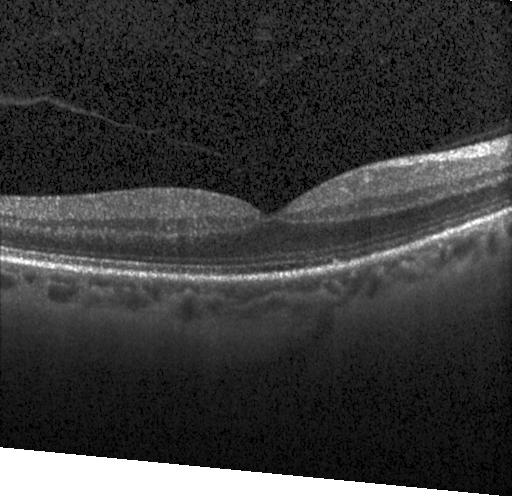

Spectral-domain optical coherence tomography, fovea-centered, Heidelberg Spectralis OCT system, retinal OCT B-scan — The scan shows no choroidal neovascularization, diabetic macular edema, or drusen.